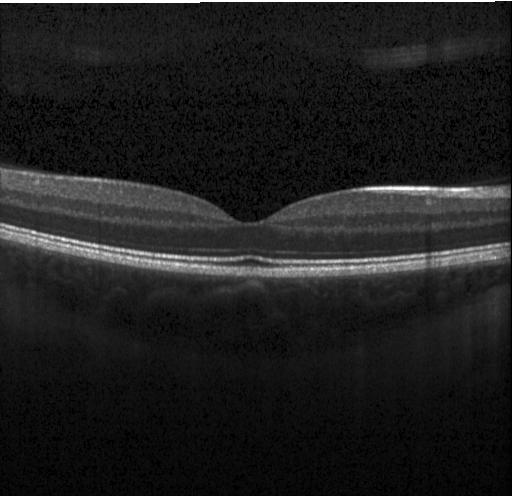
OCT B-scan showing no CNV, DME, or drusen.